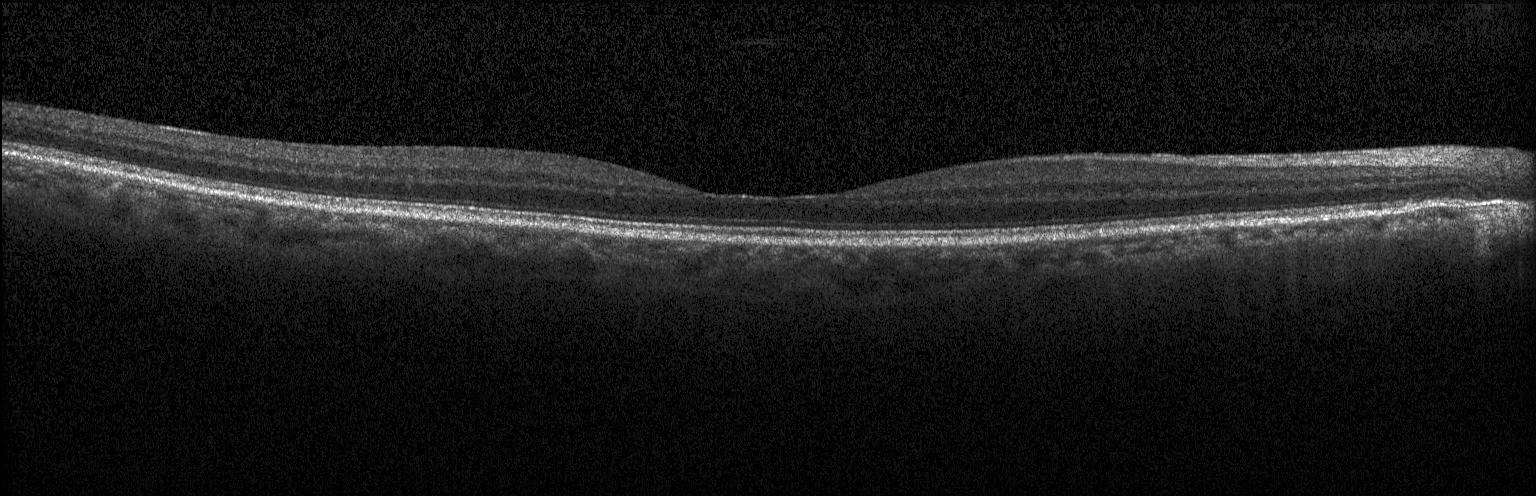

Diagnosis: no choroidal neovascularization, diabetic macular edema, or drusen.